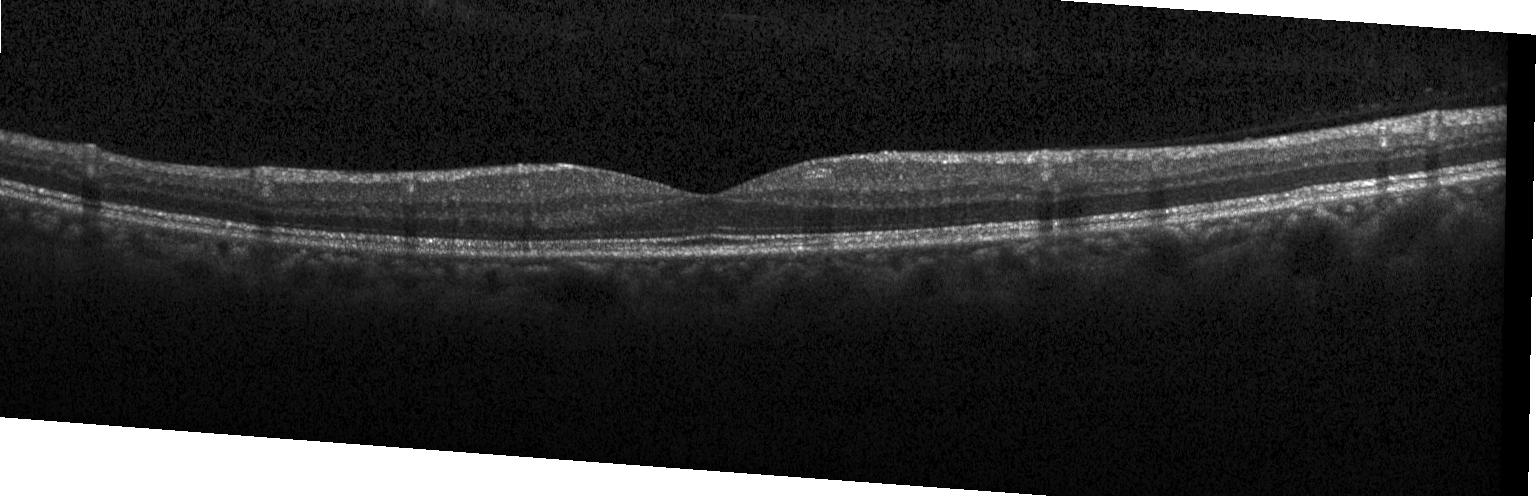 OCT B-scan showing no choroidal neovascularization, diabetic macular edema, or drusen.